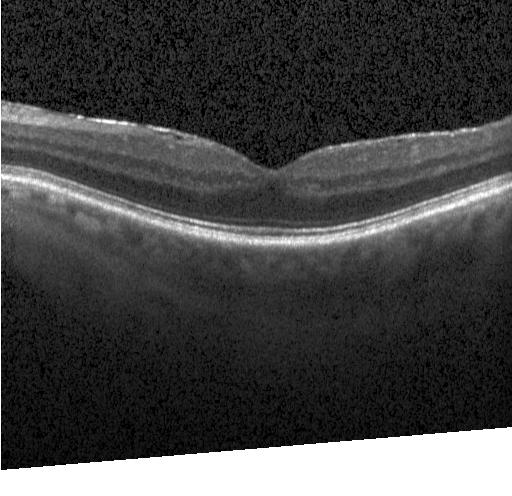

Retinal OCT cross-section
Finding: neither choroidal neovascularization, diabetic macular edema, nor drusen.